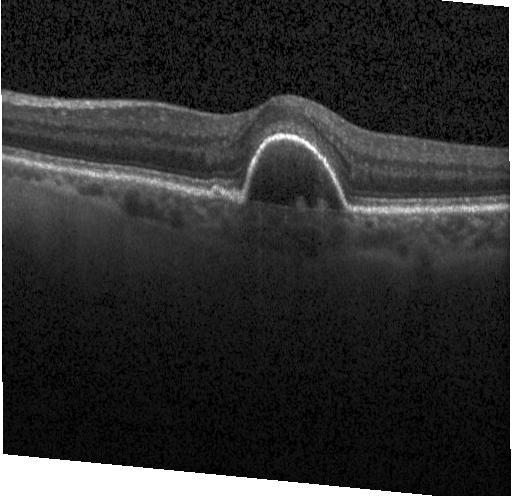 Spectral-domain OCT B-scan: a choroidal neovascular membrane.